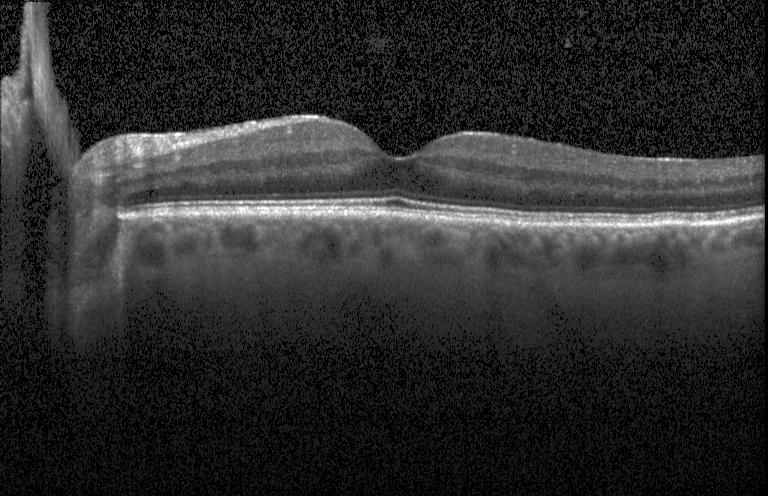

Heidelberg Spectralis OCT system, retinal OCT B-scan, SD-OCT. Neither choroidal neovascularization, diabetic macular edema, nor drusen.